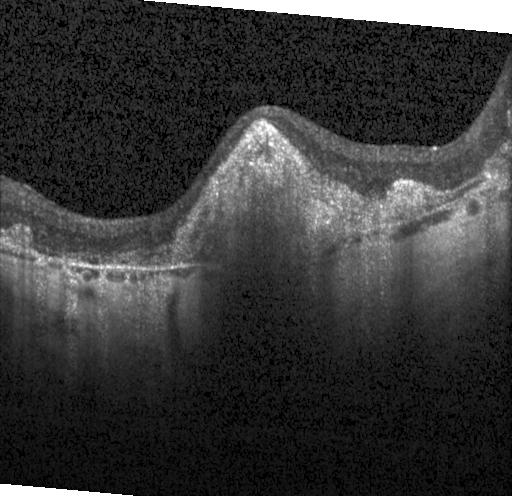 Spectral-domain OCT; centered on the fovea; optical coherence tomography B-scan — Assessment: a choroidal neovascular membrane.